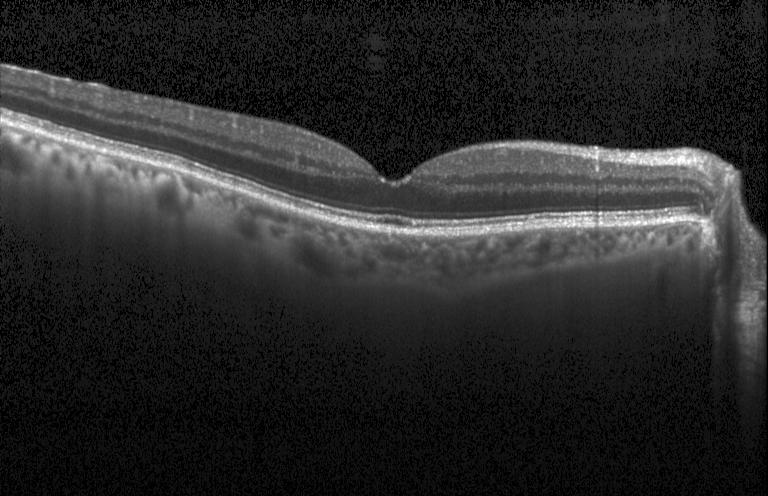 Optical coherence tomography B-scan
Impression: no choroidal neovascularization, no diabetic macular edema, and no drusen.